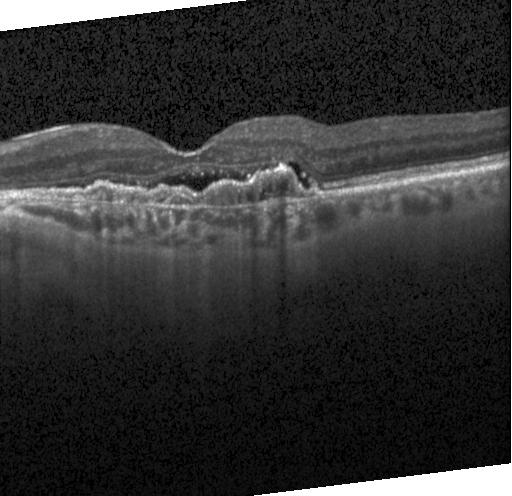
Centered on the fovea. Instrument: Heidelberg Spectralis. SD-OCT. Retinal OCT cross-section
Finding: CNV.